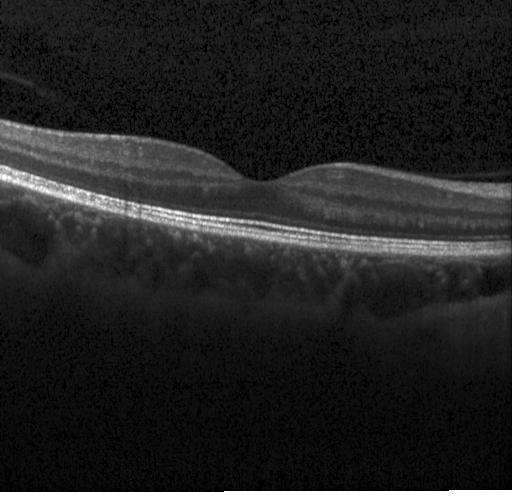

Through the macula; SD-OCT; acquired on a Heidelberg Spectralis; OCT line scan.
Finding: no choroidal neovascularization, no diabetic macular edema, and no drusen.